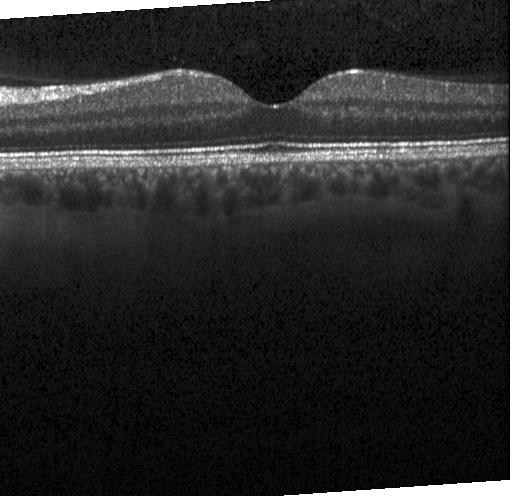
OCT B-scan · Heidelberg Spectralis · SD-OCT · fovea-centered — Impression: no evidence of choroidal neovascularization, diabetic macular edema, or drusen.